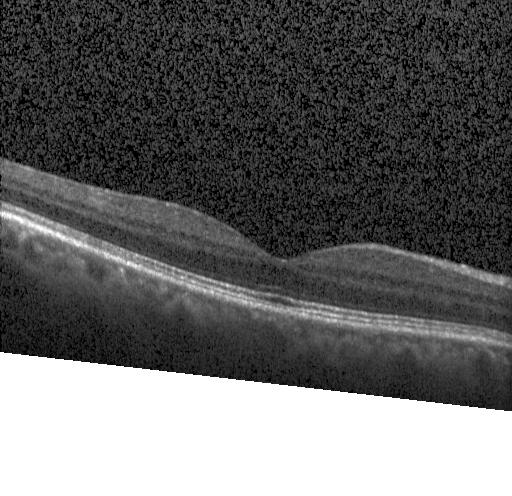 OCT finding: no choroidal neovascularization, no diabetic macular edema, and no drusen.